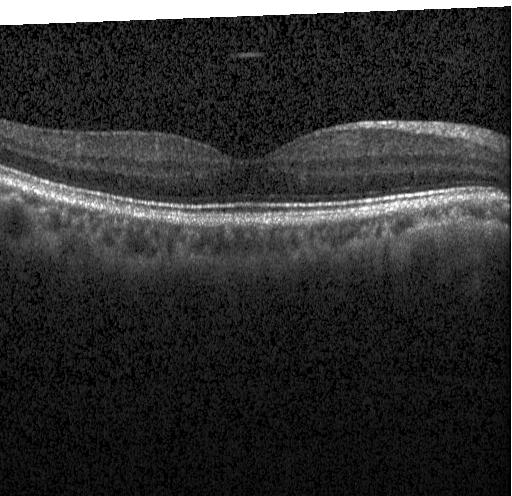
OCT finding: neither choroidal neovascularization, diabetic macular edema, nor drusen.